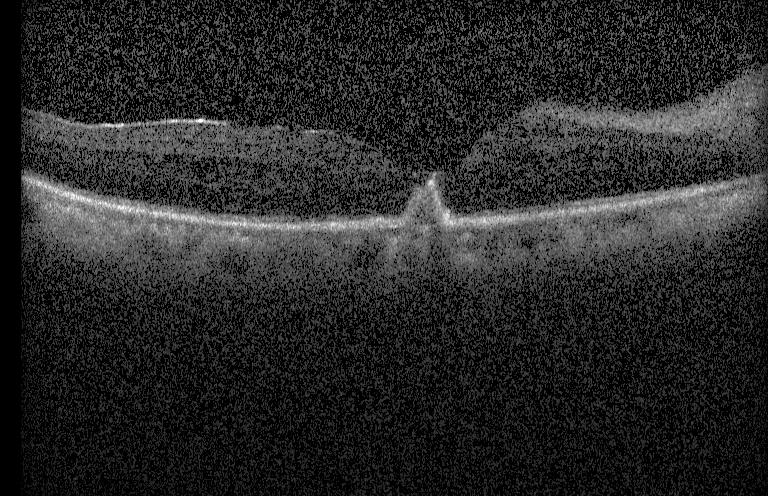

Spectral-domain OCT · Heidelberg Spectralis · centered on the fovea · optical coherence tomography B-scan — A choroidal neovascular membrane.